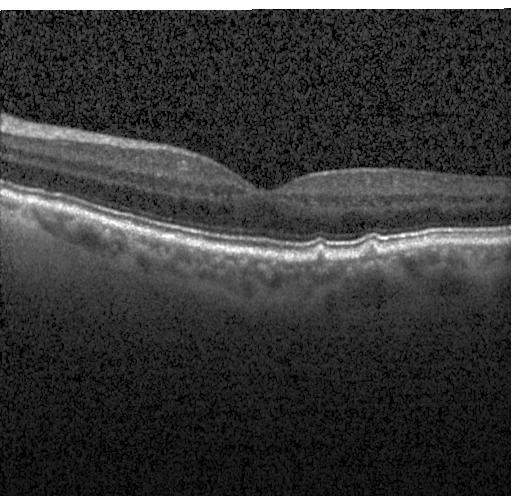

Spectral-domain OCT, retinal OCT B-scan. Sub-RPE drusenoid deposits.